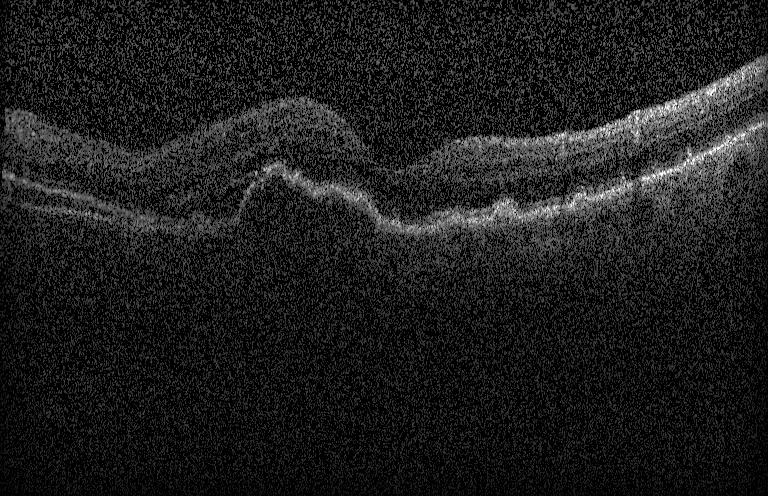

OCT B-scan showing choroidal neovascularization.